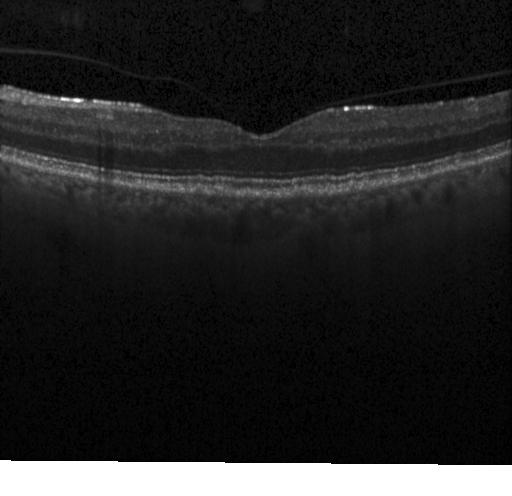
Heidelberg Spectralis OCT system, retinal OCT B-scan, horizontal scan through the fovea.
Finding: drusen.